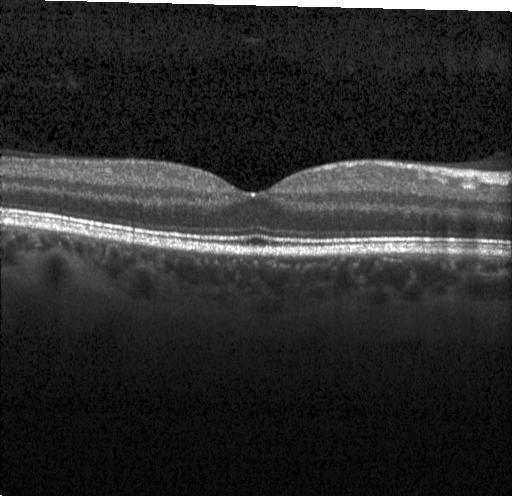
Acquired on a Heidelberg Spectralis; optical coherence tomography B-scan
OCT finding: no CNV, no DME, and no drusen.